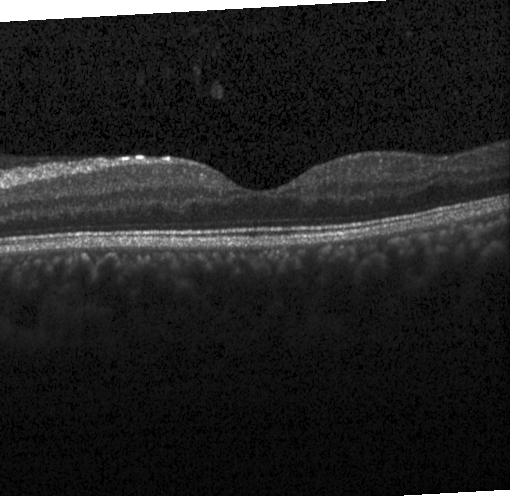

Spectral-domain OCT; optical coherence tomography scan
The scan shows no evidence of CNV, DME, or drusen.